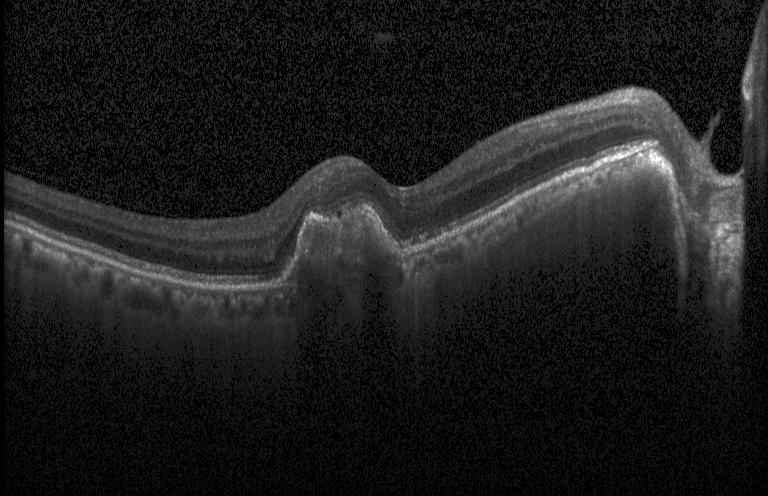

Instrument: Heidelberg Spectralis, through the macula, retinal OCT B-scan
Diagnosis: choroidal neovascularization.